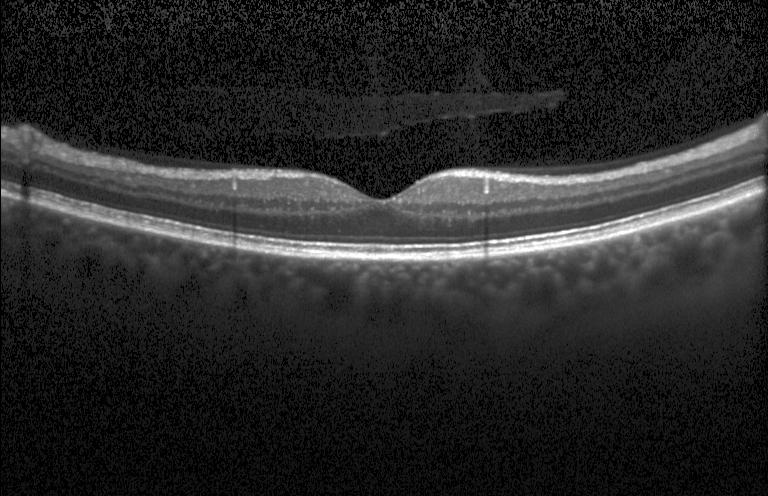

Heidelberg Spectralis · retinal OCT B-scan — The scan shows no choroidal neovascularization, no diabetic macular edema, and no drusen.